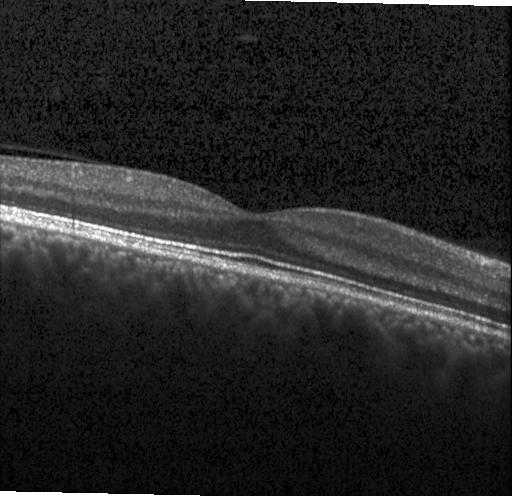 Instrument: Heidelberg Spectralis; retinal OCT B-scan; fovea-centered.
The scan shows no evidence of CNV, DME, or drusen.